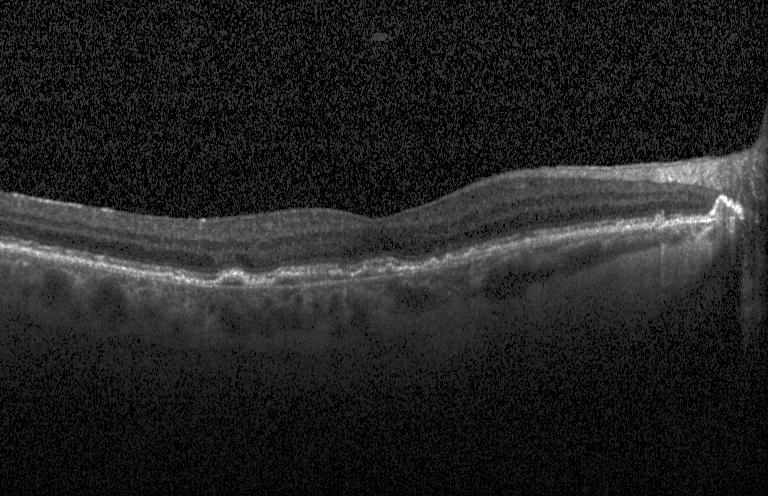 Retinal OCT cross-section. OCT finding: a choroidal neovascular membrane.